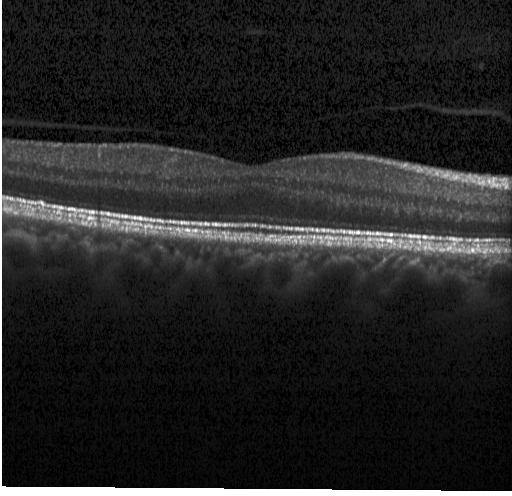
Spectral-domain OCT. Retinal OCT cross-section. Fovea-centered.
Macular OCT: no evidence of CNV, DME, or drusen.